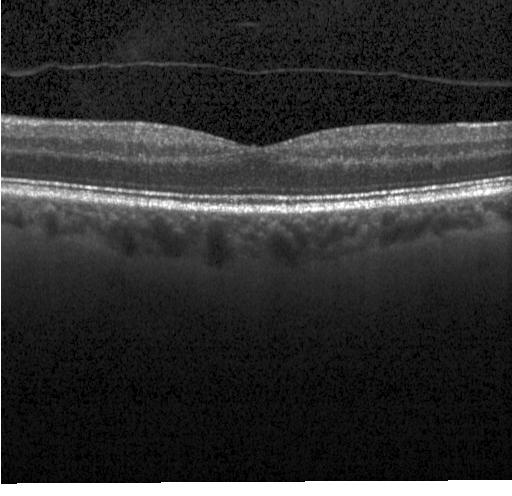 The scan shows no choroidal neovascularization, diabetic macular edema, or drusen.